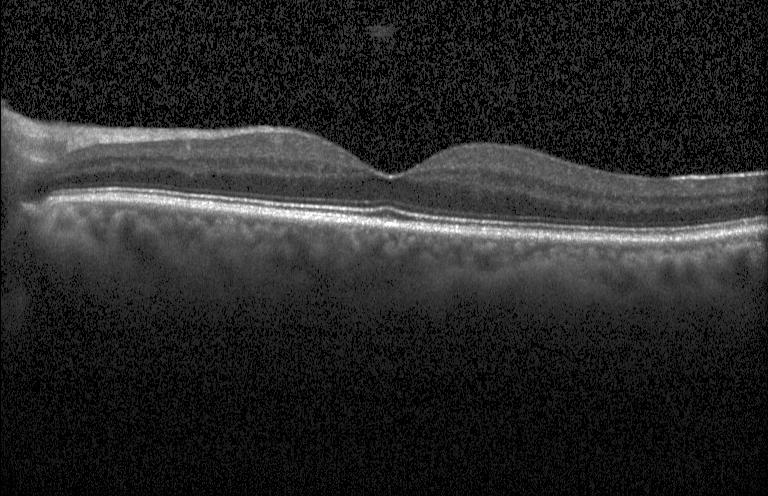 The scan shows no evidence of choroidal neovascularization, diabetic macular edema, or drusen.